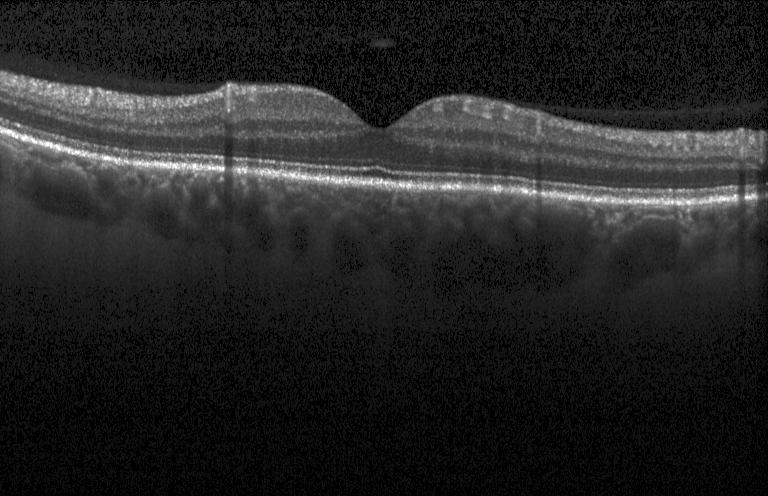 Assessment: neither choroidal neovascularization, diabetic macular edema, nor drusen.